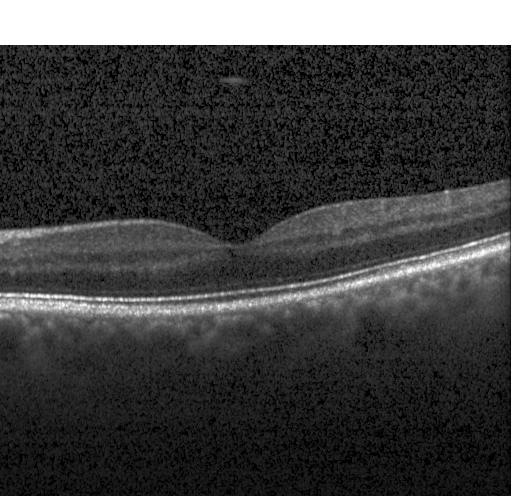 Diagnosis: no evidence of CNV, DME, or drusen.